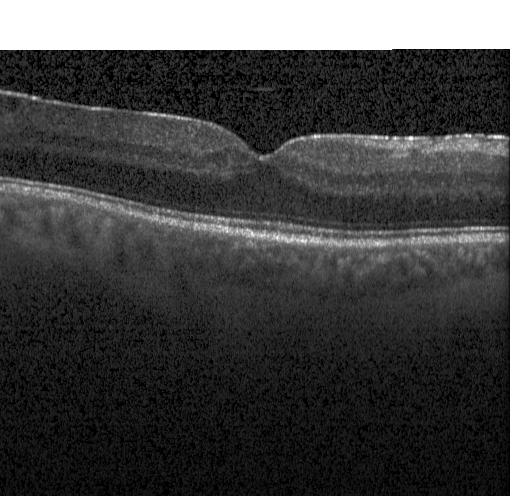

Optical coherence tomography scan.
Diagnosis: no CNV, no DME, and no drusen.